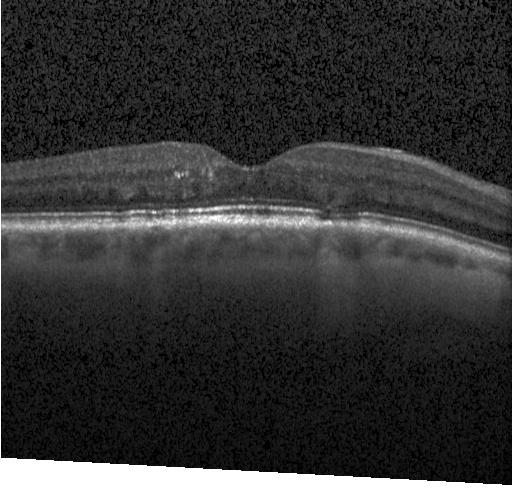

Spectral-domain OCT. Acquired on a Heidelberg Spectralis. Centered on the fovea. OCT B-scan
Finding: diabetic macular edema (DME).